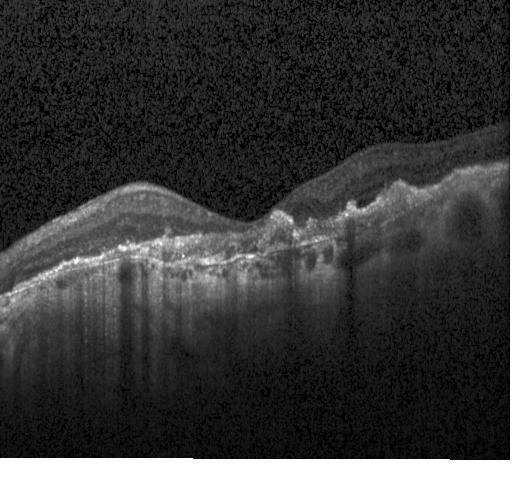

OCT B-scan
Impression: CNV.